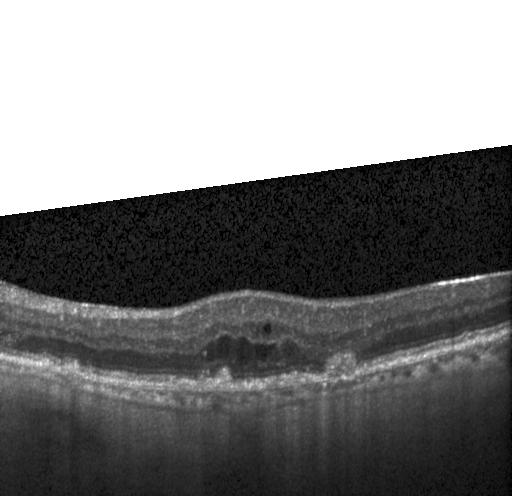 OCT scan showing a choroidal neovascular membrane.